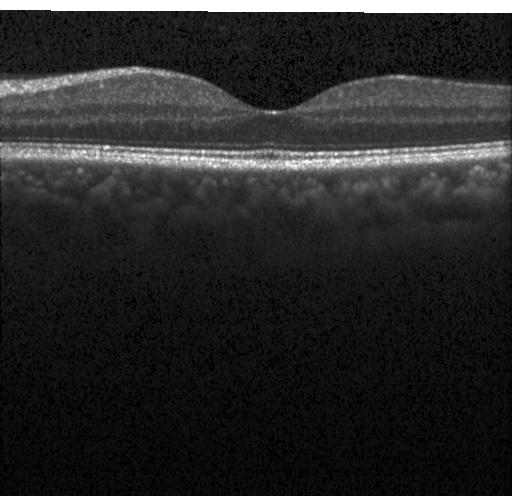 SD-OCT · through the macula · optical coherence tomography scan · Heidelberg Spectralis.
Impression: no CNV, DME, or drusen.